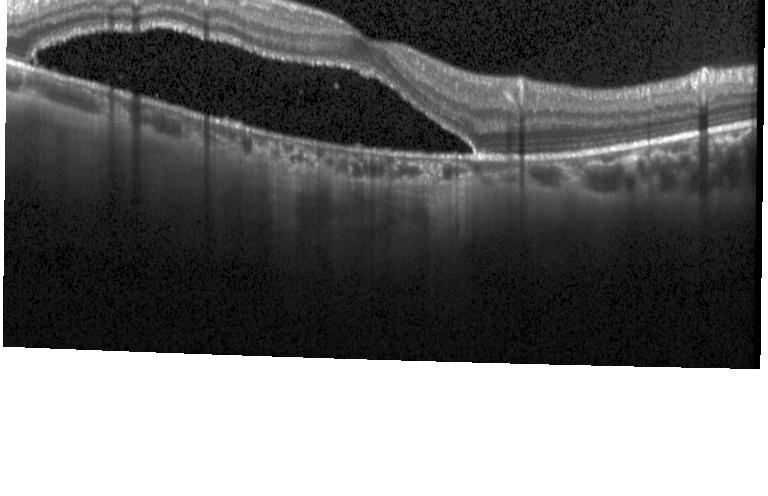
Retinal OCT B-scan
This B-scan demonstrates a choroidal neovascular membrane.